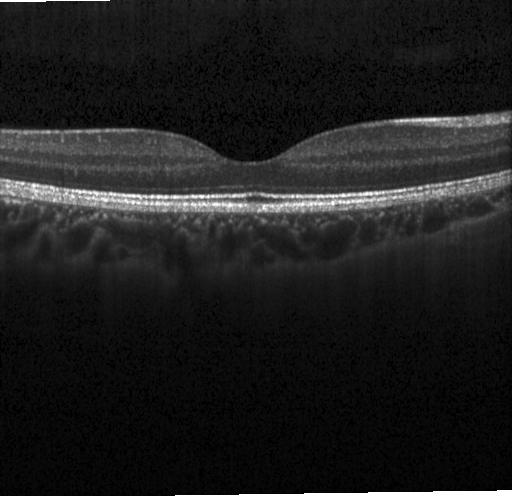 Heidelberg Spectralis OCT system. Optical coherence tomography B-scan. Spectral-domain optical coherence tomography — Finding: no choroidal neovascularization, no diabetic macular edema, and no drusen.